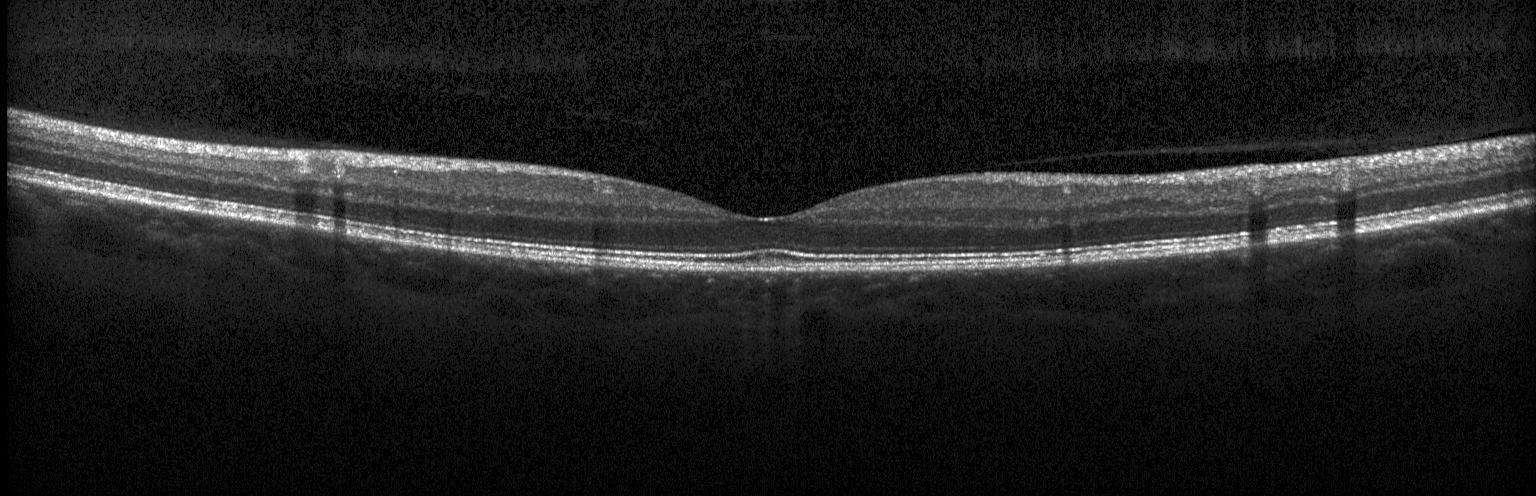 Macular scan · optical coherence tomography scan · instrument: Heidelberg Spectralis. Impression: no choroidal neovascularization, no diabetic macular edema, and no drusen.